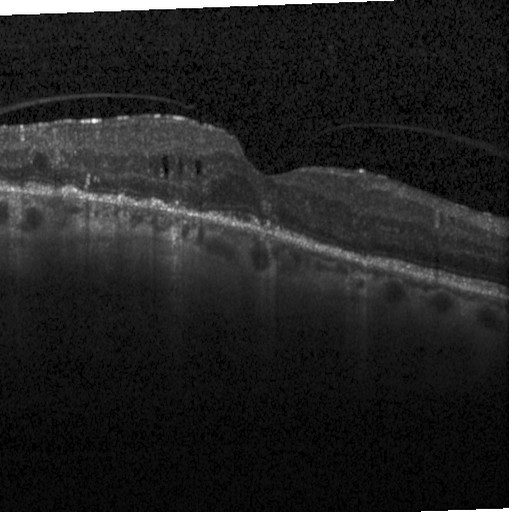
Optical coherence tomography B-scan
Assessment: DME.